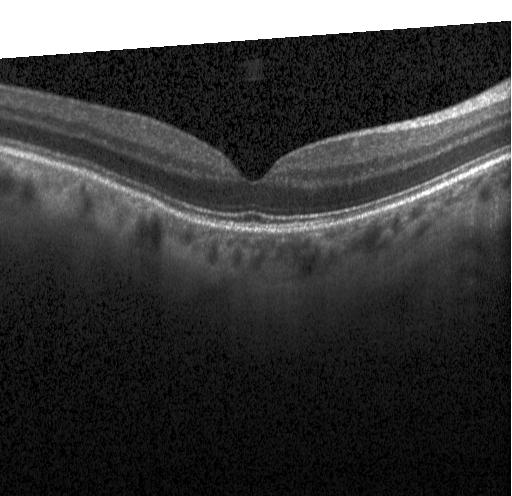 Retinal OCT B-scan. Acquired on a Heidelberg Spectralis. Centered on the fovea. Spectral-domain OCT. OCT finding: no CNV, DME, or drusen.